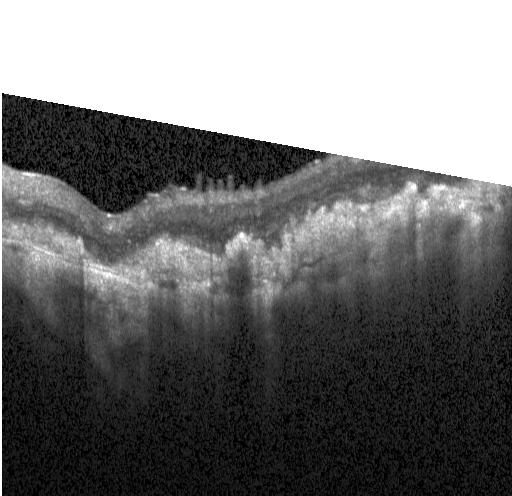 OCT B-scan. Spectral-domain optical coherence tomography — Finding: a choroidal neovascular membrane.